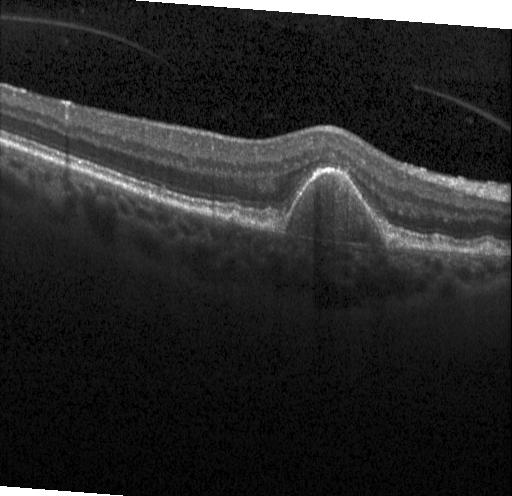

Heidelberg Spectralis OCT system; through the macula; spectral-domain optical coherence tomography; optical coherence tomography B-scan — Diagnosis: choroidal neovascularization (CNV).